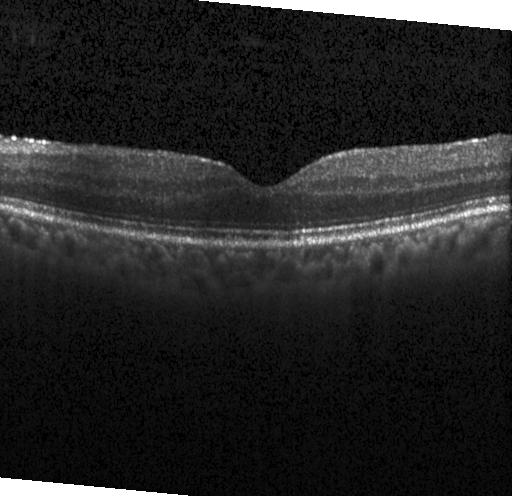

Finding: neither choroidal neovascularization, diabetic macular edema, nor drusen.